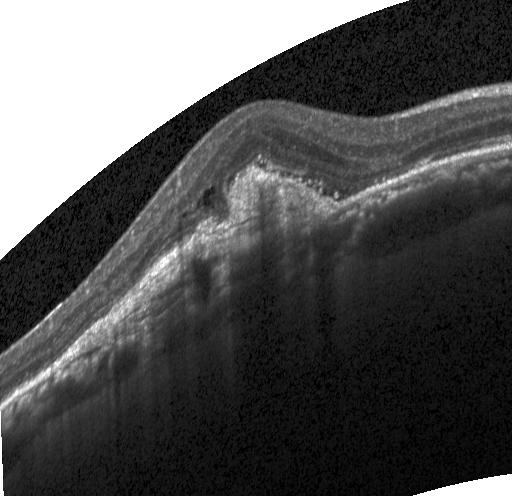
Finding: a choroidal neovascular membrane.